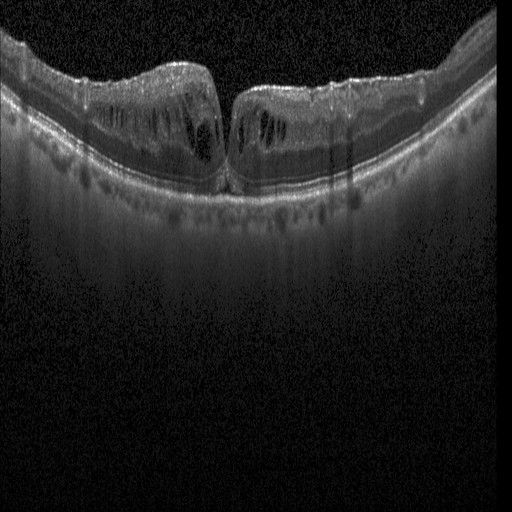 Diagnosis: diabetic macular edema (DME).